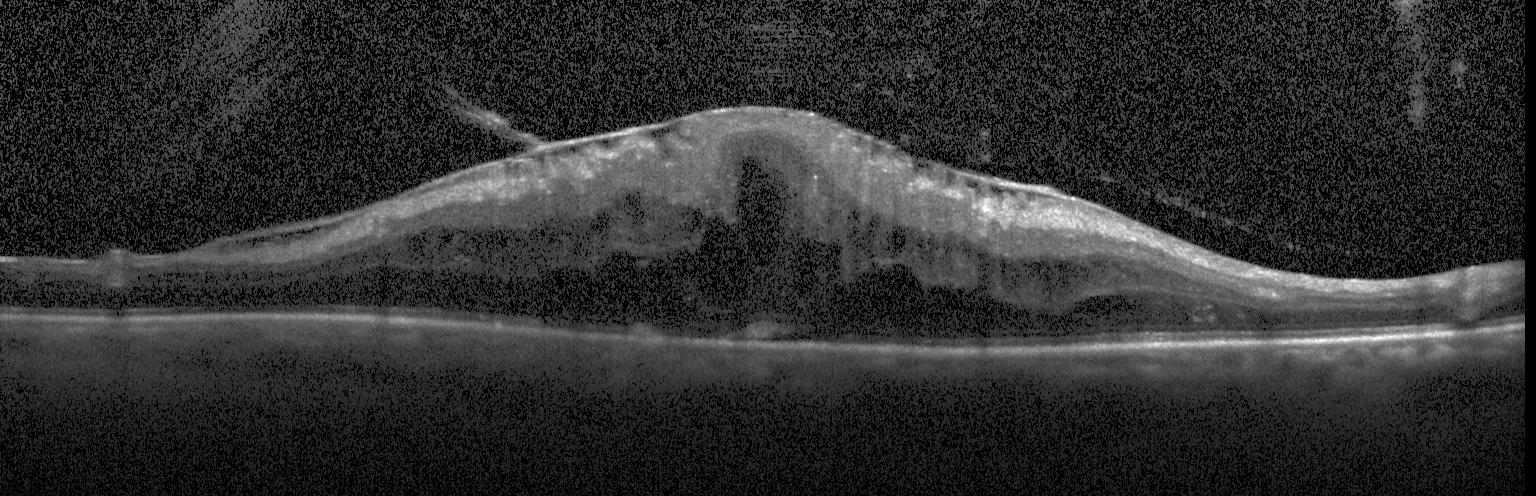
Optical coherence tomography scan
Assessment: diabetic macular edema (DME).